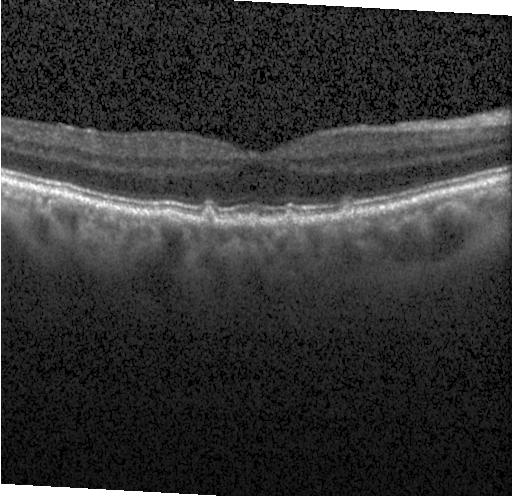 Assessment: sub-RPE drusenoid deposits.